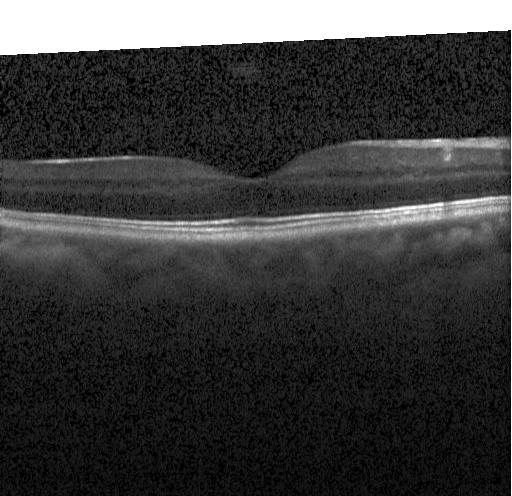
The scan shows no CNV, DME, or drusen.